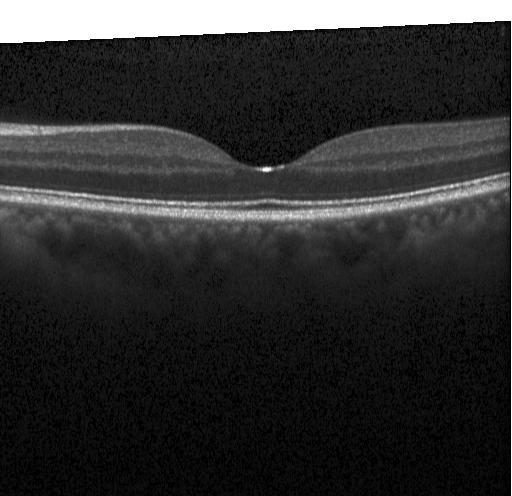 Macular OCT demonstrating no evidence of choroidal neovascularization, diabetic macular edema, or drusen.